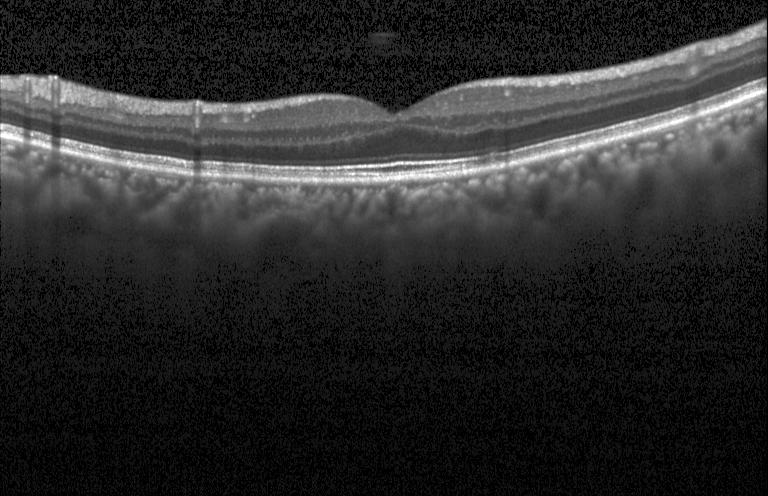
Assessment: no evidence of CNV, DME, or drusen.